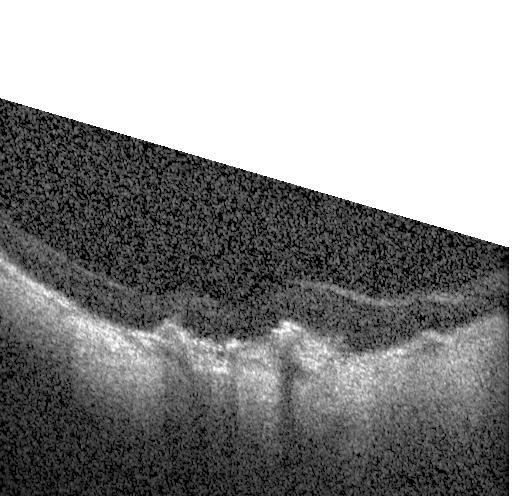
Assessment: a choroidal neovascular membrane.